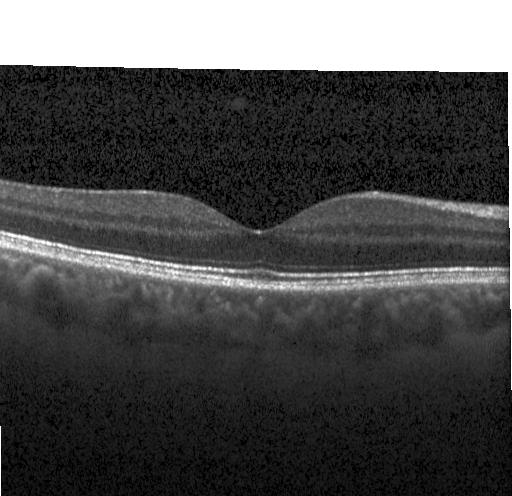 Spectral-domain OCT. Fovea-centered. Heidelberg Spectralis. Retinal OCT cross-section — No choroidal neovascularization, diabetic macular edema, or drusen.